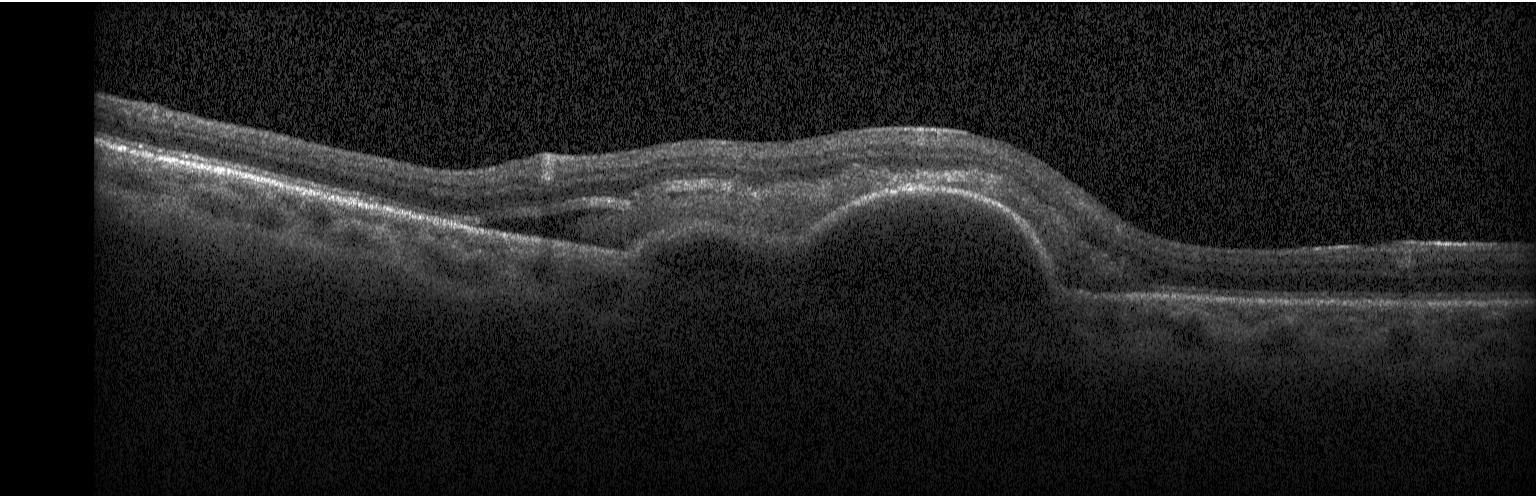

SD-OCT · fovea-centered · retinal OCT cross-section · acquired on a Heidelberg Spectralis. Diagnosis: choroidal neovascularization.